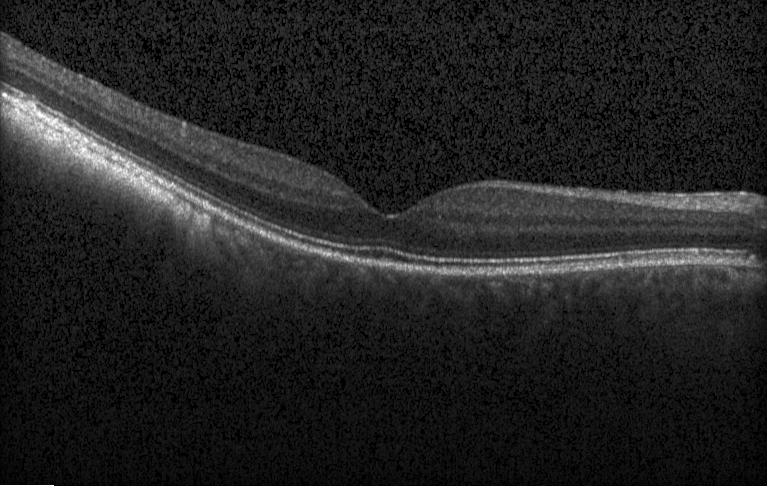
OCT finding: multiple drusen.